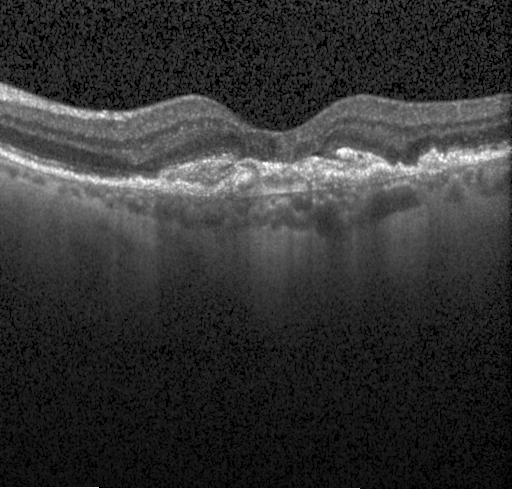 Retinal OCT cross-section showing a choroidal neovascular membrane.